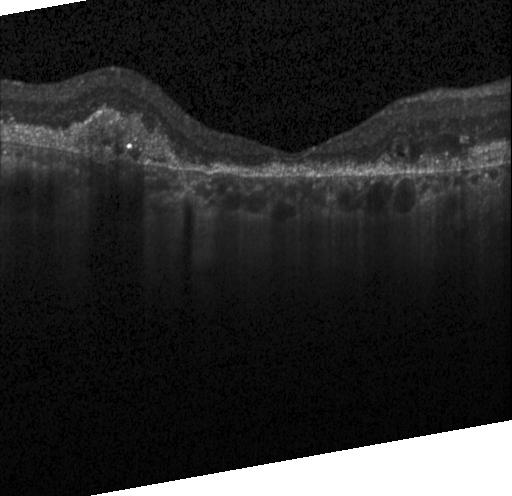 OCT finding: a choroidal neovascular membrane.